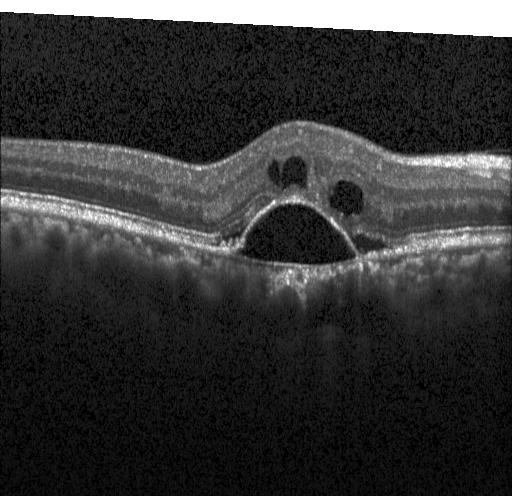
OCT B-scan showing a choroidal neovascular membrane.